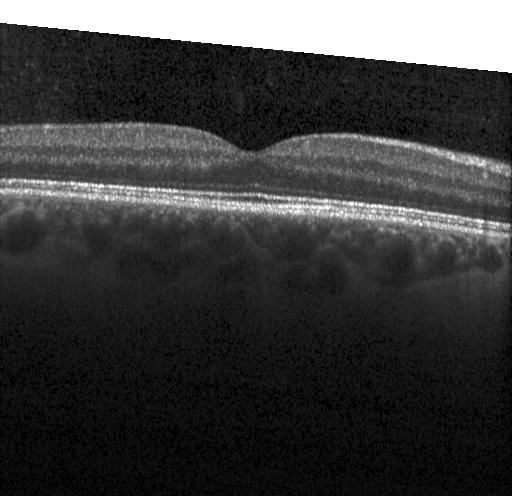 OCT line scan — Assessment: no evidence of choroidal neovascularization, diabetic macular edema, or drusen.